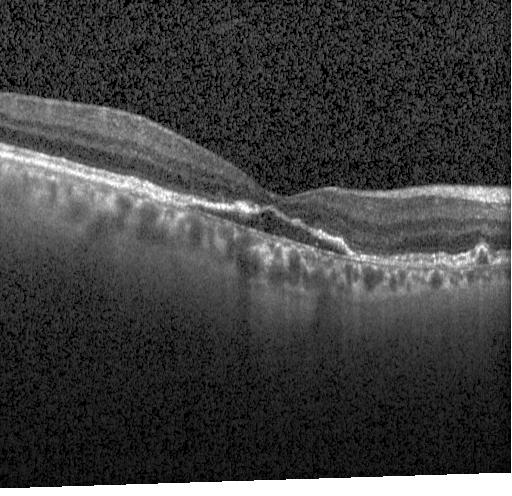
Macular scan · spectral-domain OCT · OCT line scan.
CNV.